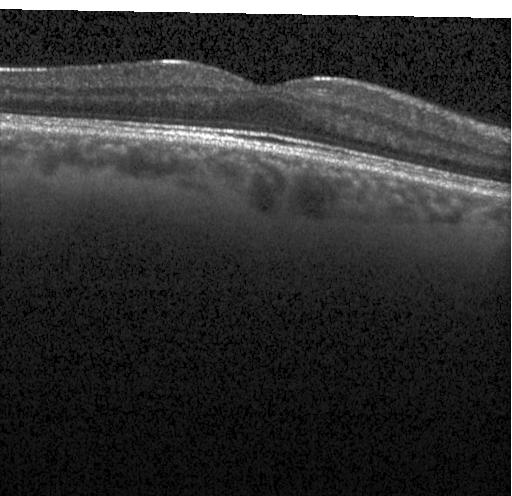 Finding: no choroidal neovascularization, diabetic macular edema, or drusen.